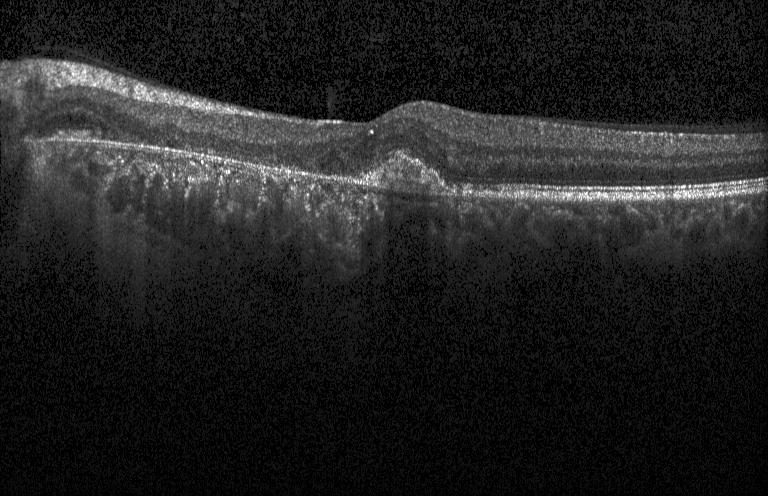
Optical coherence tomography B-scan. SD-OCT
Impression: a choroidal neovascular membrane.